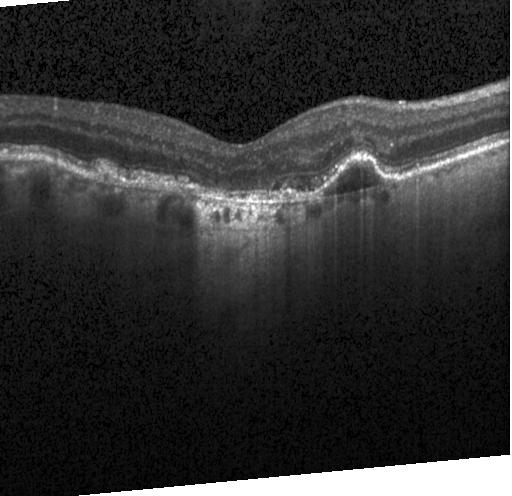
Through the macula, optical coherence tomography scan, spectral-domain optical coherence tomography, acquired on a Heidelberg Spectralis.
Macular OCT: a choroidal neovascular membrane.